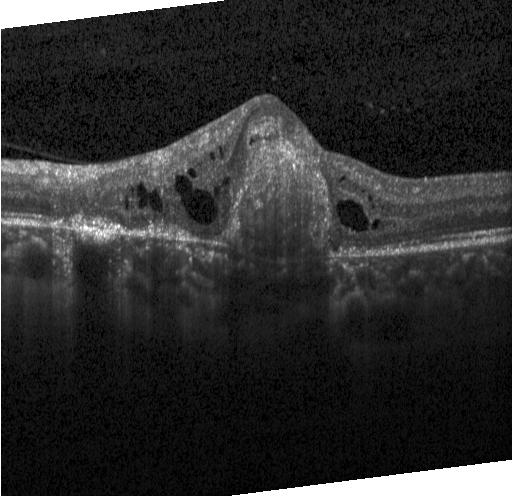
OCT B-scan. CNV.